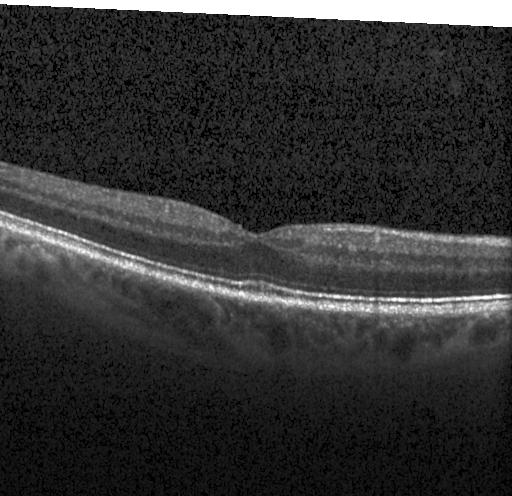 Dx: no choroidal neovascularization, no diabetic macular edema, and no drusen.